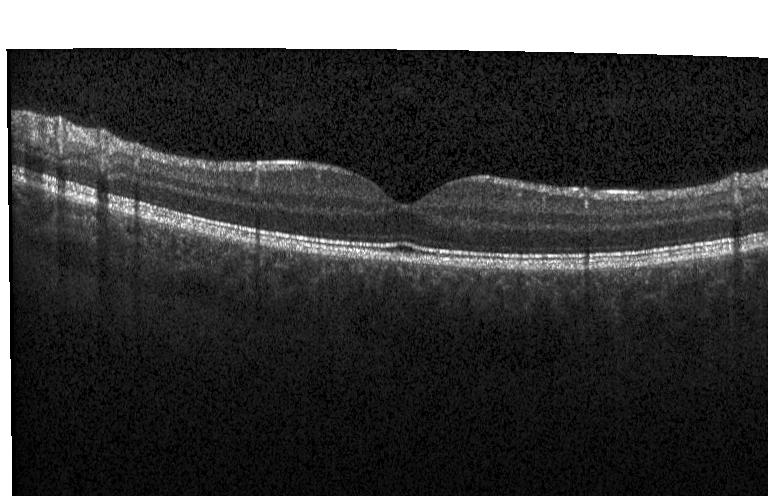 OCT B-scan — Diagnosis: neither choroidal neovascularization, diabetic macular edema, nor drusen.